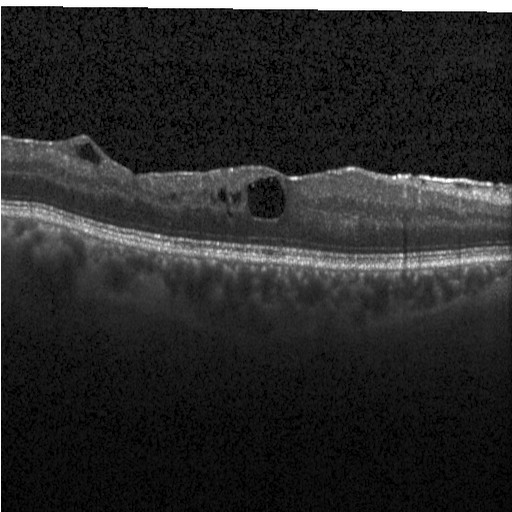

Acquired on a Heidelberg Spectralis, OCT B-scan.
Dx: DME.